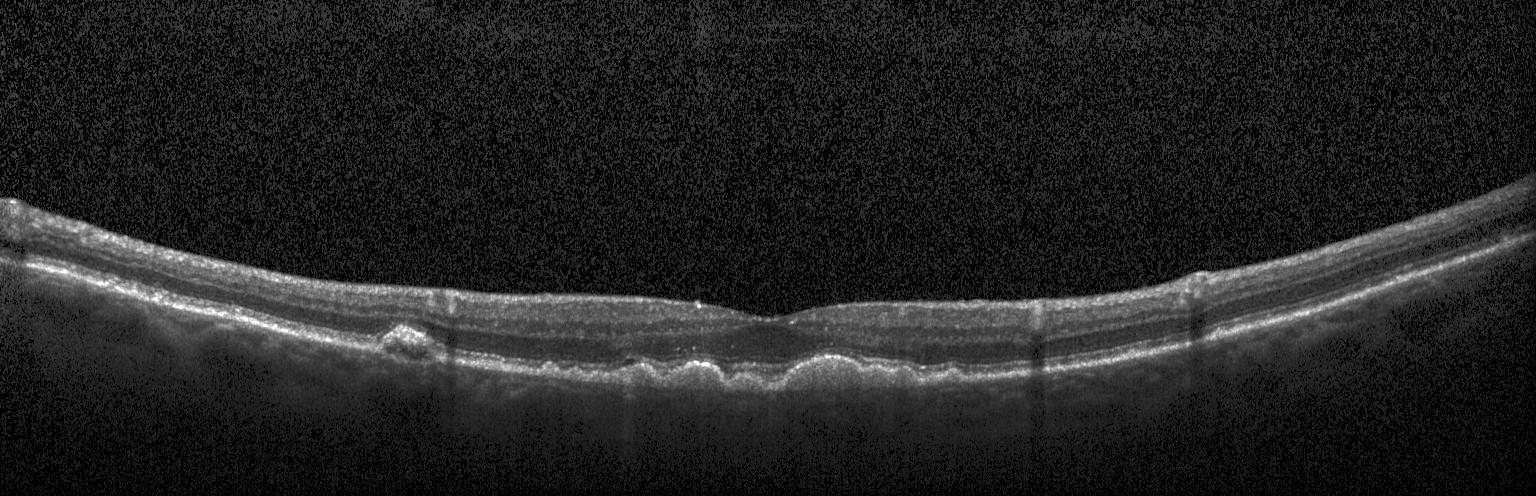 Impression: drusen.